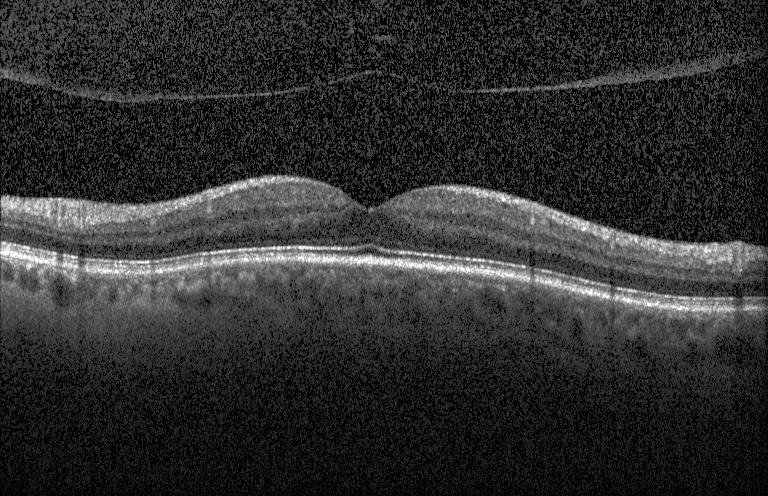

Acquired on a Heidelberg Spectralis. Retinal OCT cross-section. Through the macula
The scan shows no CNV, no DME, and no drusen.